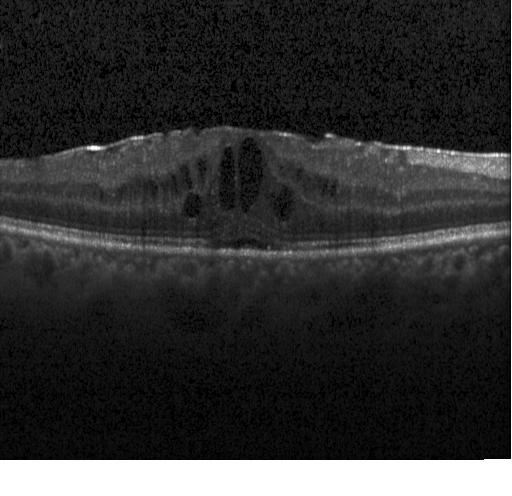
Centered on the fovea, instrument: Heidelberg Spectralis, spectral-domain OCT, optical coherence tomography B-scan
Impression: DME.